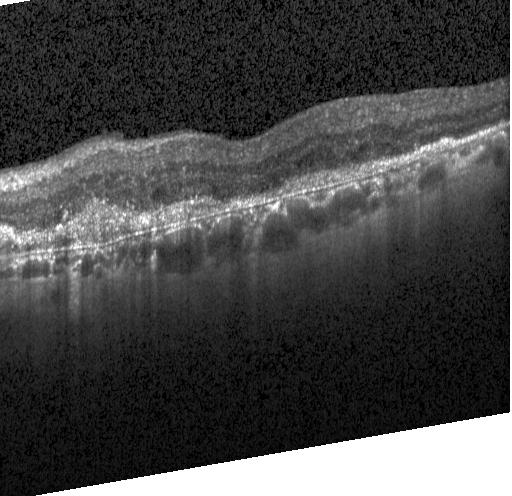

SD-OCT; OCT B-scan. Finding: CNV.